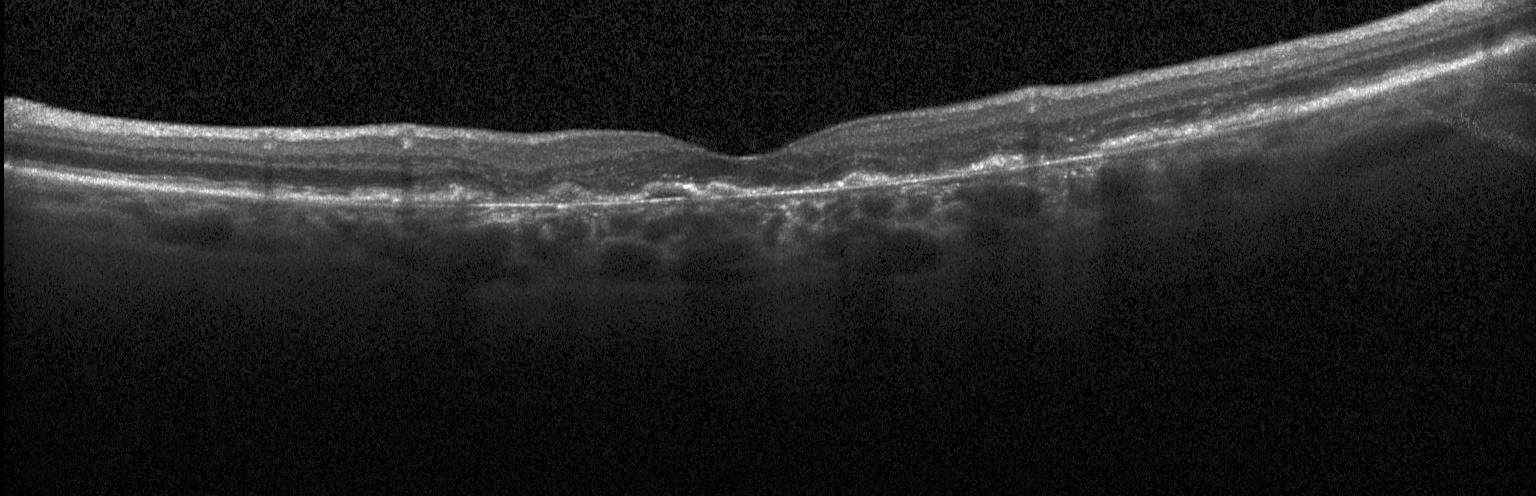
OCT line scan; SD-OCT
Diagnosis: choroidal neovascularization.